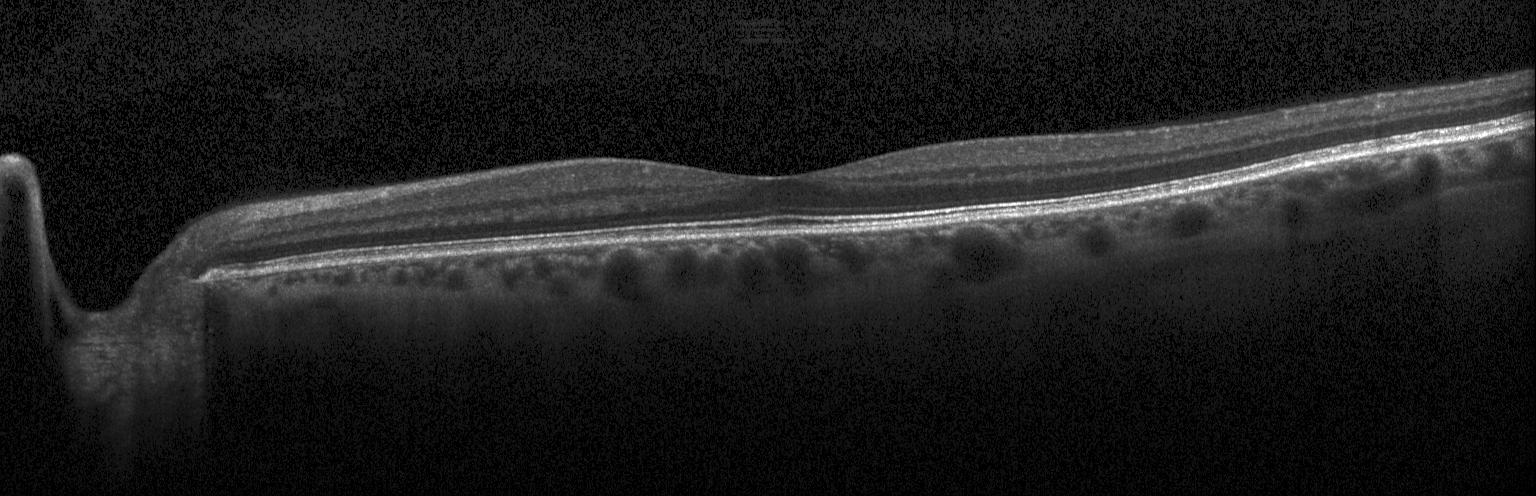

Through the macula. OCT line scan. Spectral-domain optical coherence tomography. Acquired on a Heidelberg Spectralis — Macular OCT: no choroidal neovascularization, diabetic macular edema, or drusen.